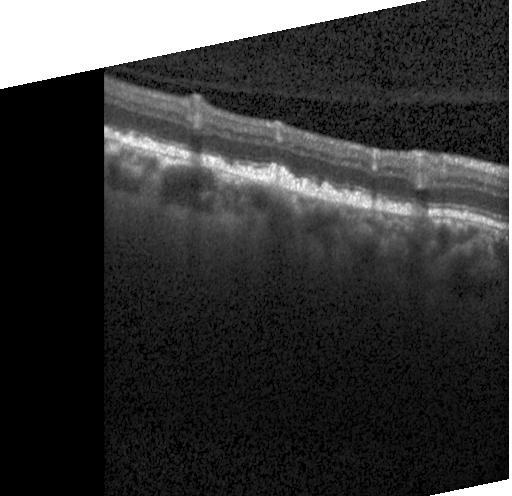

Macular scan. Spectral-domain optical coherence tomography. Acquired on a Heidelberg Spectralis. OCT line scan
Assessment: multiple drusen.